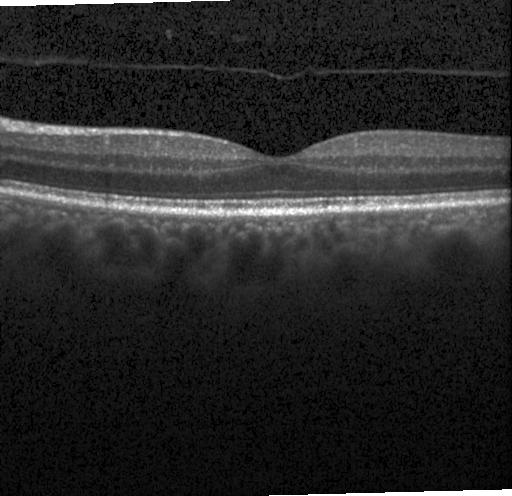

Macular OCT demonstrating no evidence of choroidal neovascularization, diabetic macular edema, or drusen.